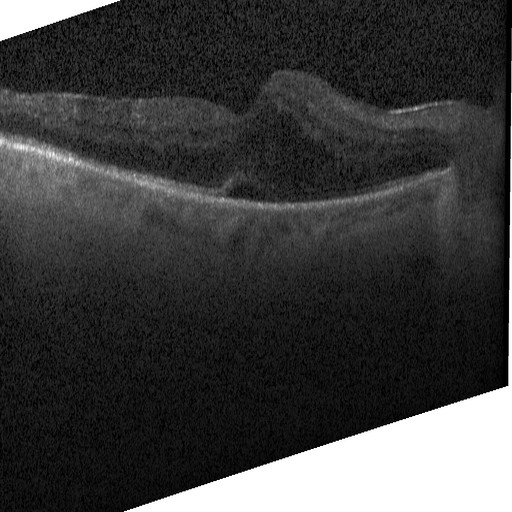

Retinal OCT cross-section showing diabetic macular edema (DME).